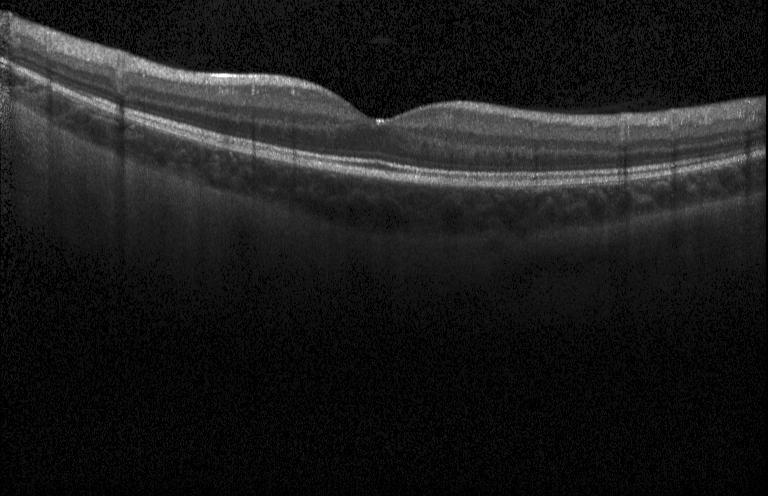 Spectral-domain OCT B-scan: no CNV, no DME, and no drusen.